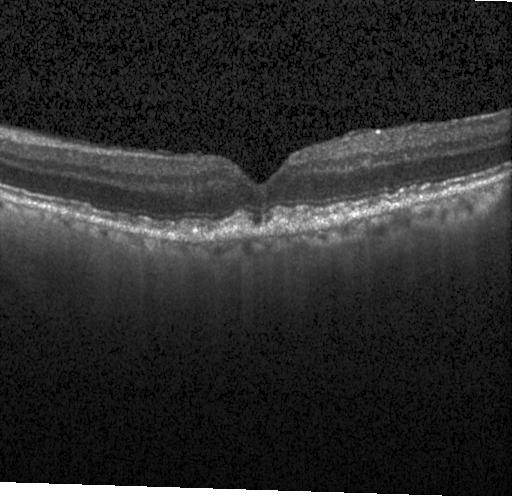 Spectral-domain optical coherence tomography. Acquired on a Heidelberg Spectralis. Fovea-centered. OCT B-scan.
Macular OCT: drusen.